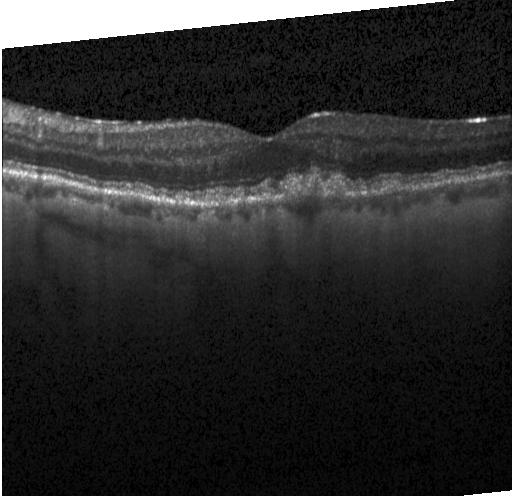

This B-scan demonstrates multiple drusen.